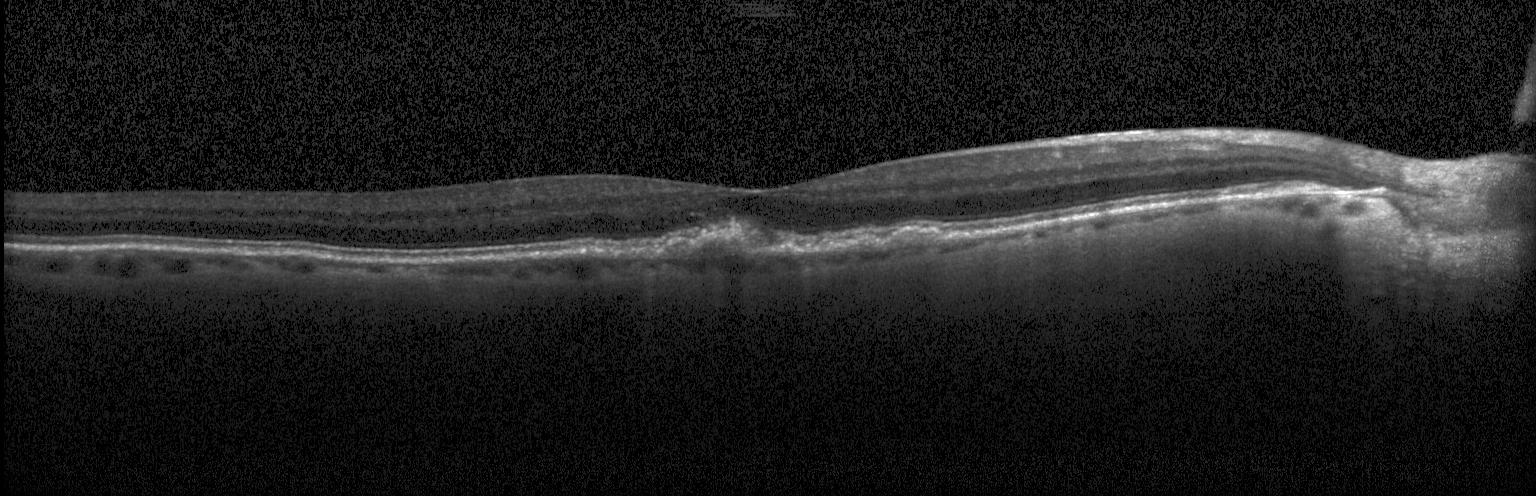

Retinal OCT B-scan — Finding: multiple drusen.